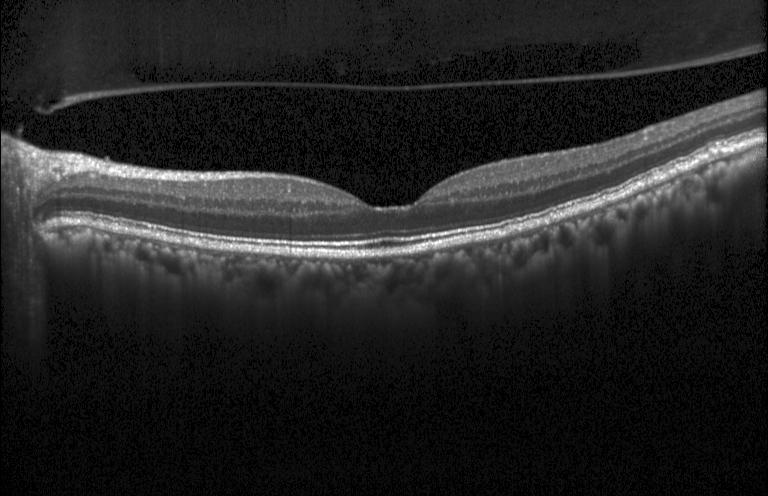

Horizontal scan through the fovea; OCT line scan
This B-scan demonstrates neither choroidal neovascularization, diabetic macular edema, nor drusen.